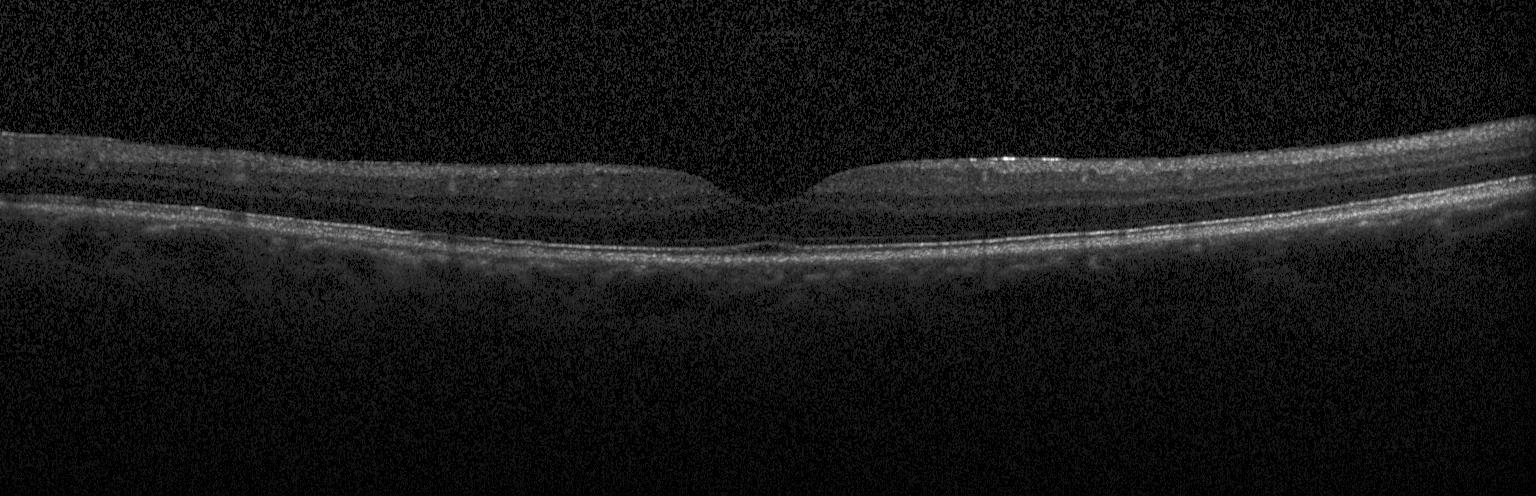

Spectral-domain optical coherence tomography, retinal OCT cross-section, macular scan.
No CNV, no DME, and no drusen.